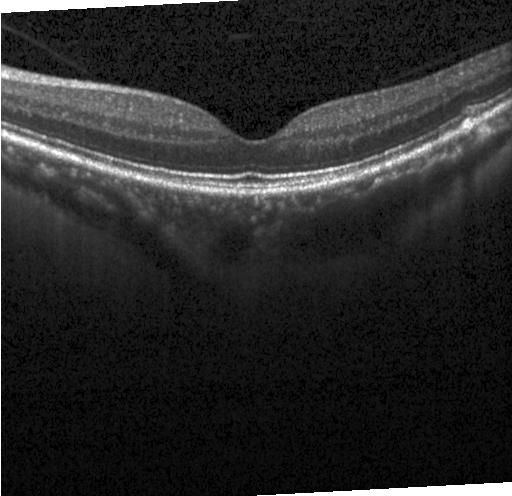
Macular OCT: no CNV, no DME, and no drusen.